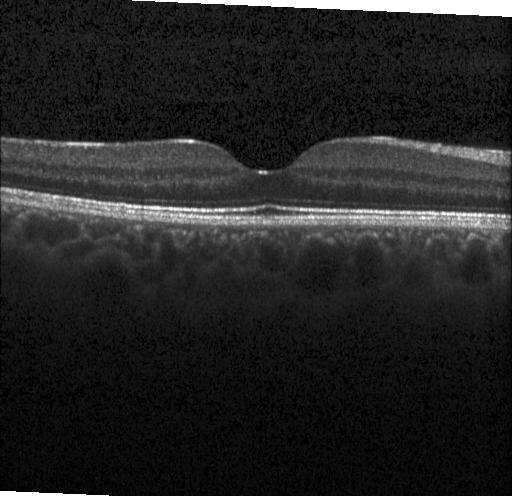
Macular OCT demonstrating no choroidal neovascularization, diabetic macular edema, or drusen.